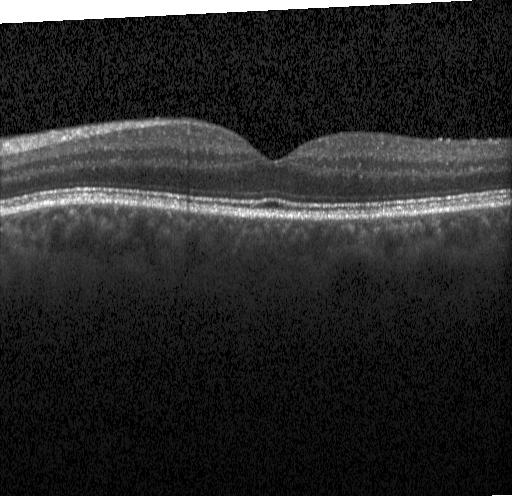 Macular OCT demonstrating no CNV, DME, or drusen.